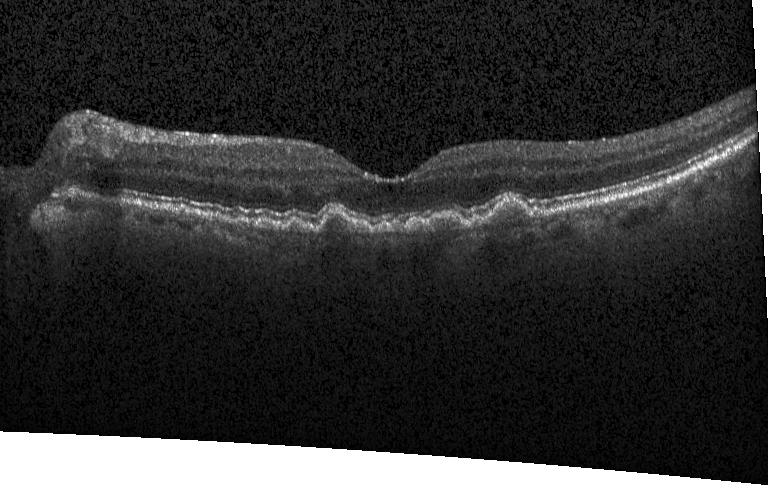 Heidelberg Spectralis OCT system; horizontal scan through the fovea; spectral-domain optical coherence tomography; OCT line scan
OCT finding: sub-RPE drusenoid deposits.